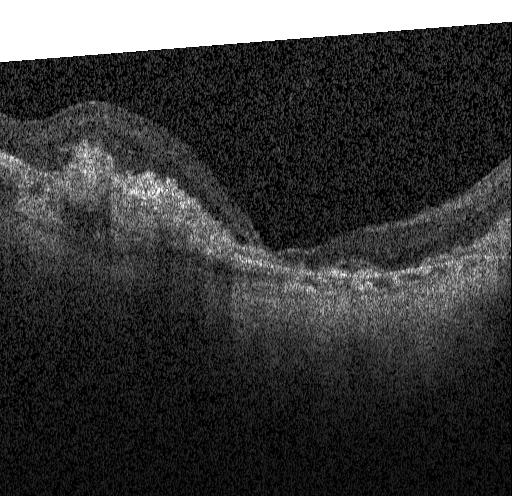
Centered on the fovea, spectral-domain OCT, retinal OCT B-scan, Heidelberg Spectralis.
OCT finding: choroidal neovascularization (CNV).